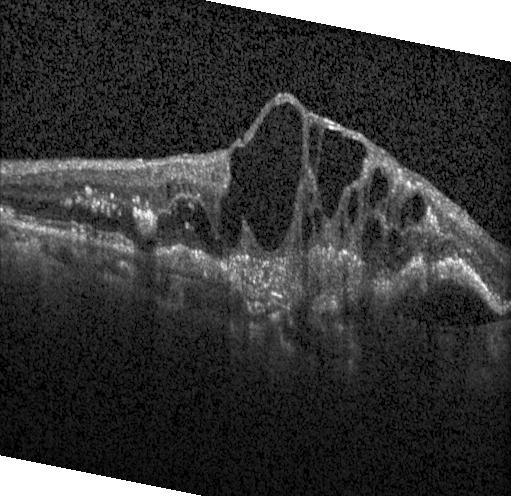 Diagnosis: a choroidal neovascular membrane.